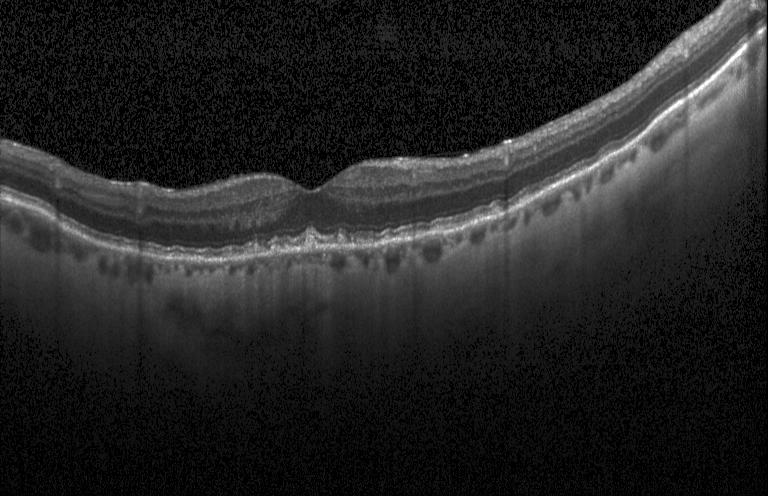

Optical coherence tomography scan · spectral-domain OCT · fovea-centered · acquired on a Heidelberg Spectralis. Finding: drusen.